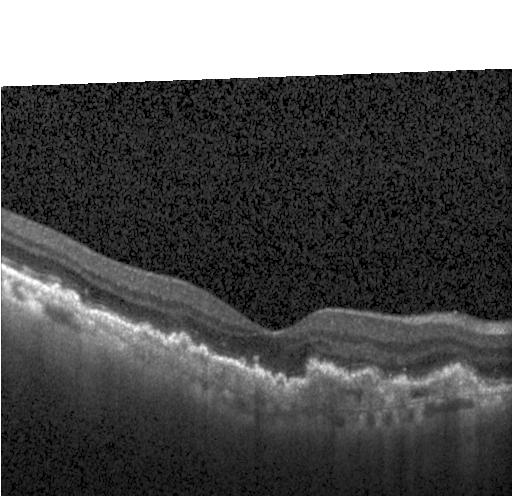 Optical coherence tomography B-scan · spectral-domain optical coherence tomography · through the macula · instrument: Heidelberg Spectralis
Macular OCT: choroidal neovascularization.